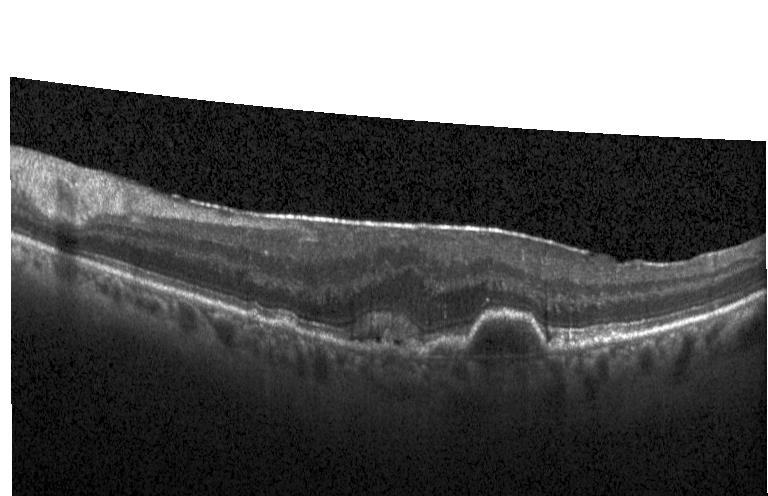 Spectral-domain OCT; through the macula; optical coherence tomography scan; Heidelberg Spectralis OCT system.
This B-scan demonstrates a choroidal neovascular membrane.